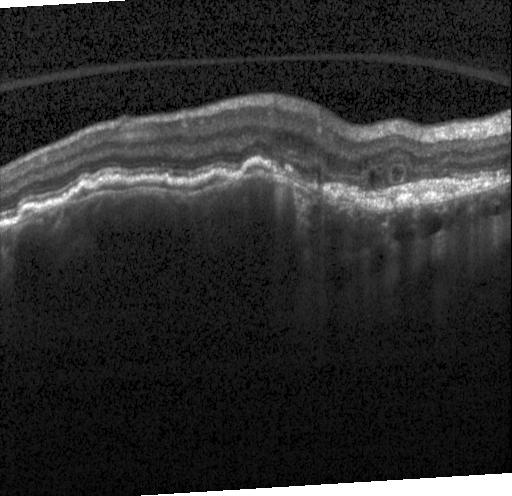 Diagnosis: CNV.